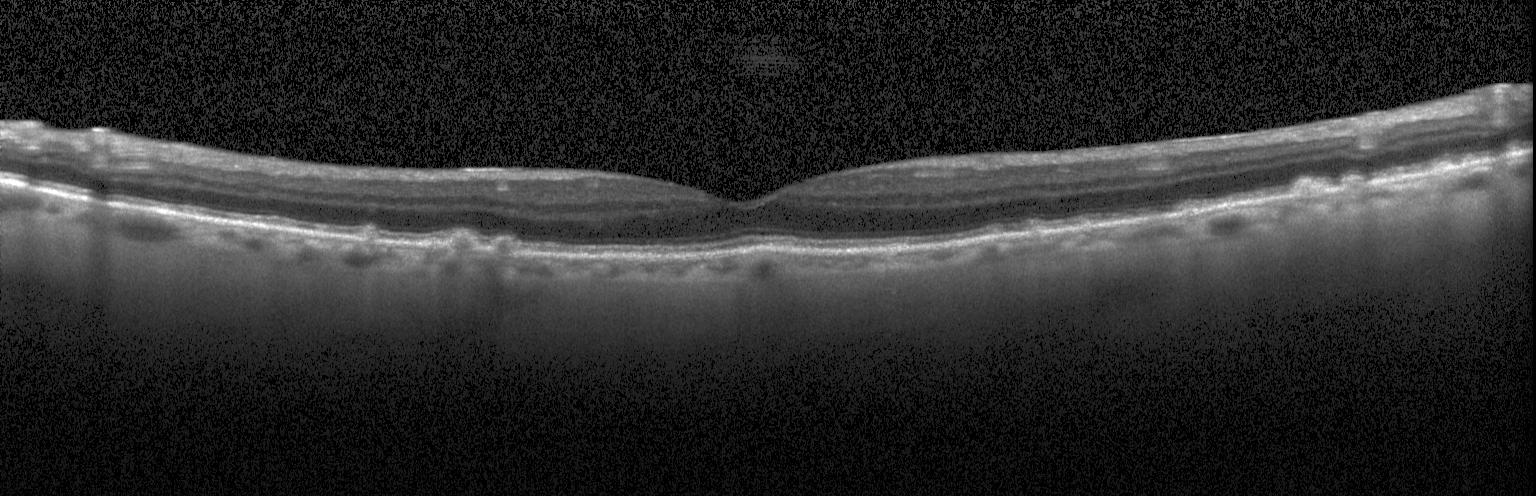
Sub-RPE drusenoid deposits.